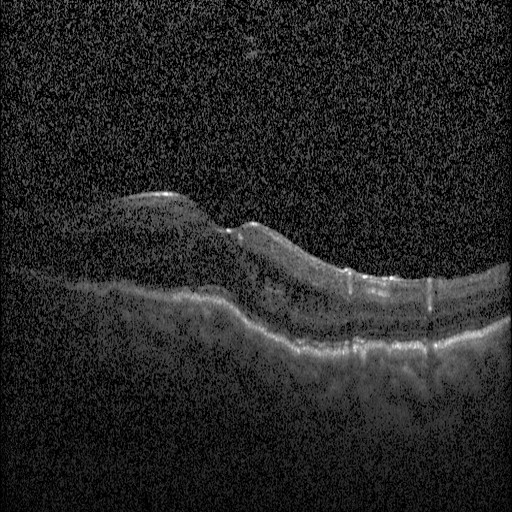
SD-OCT. Retinal OCT B-scan. Macular OCT: diabetic macular edema (DME).